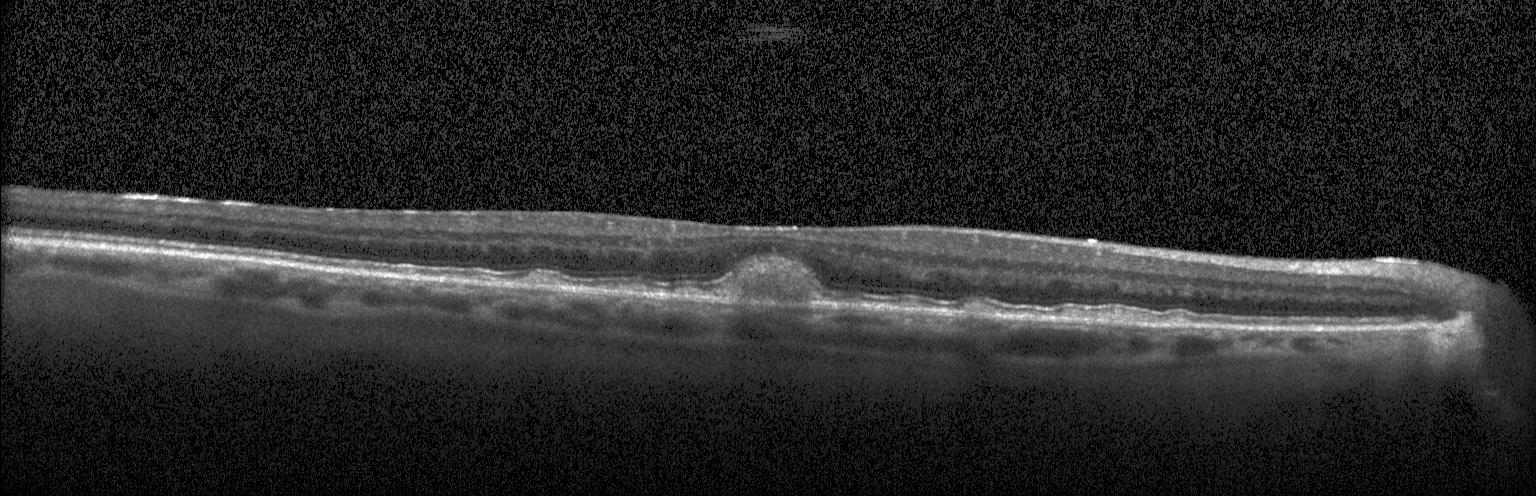 OCT line scan; macular scan; spectral-domain optical coherence tomography
This B-scan demonstrates CNV.